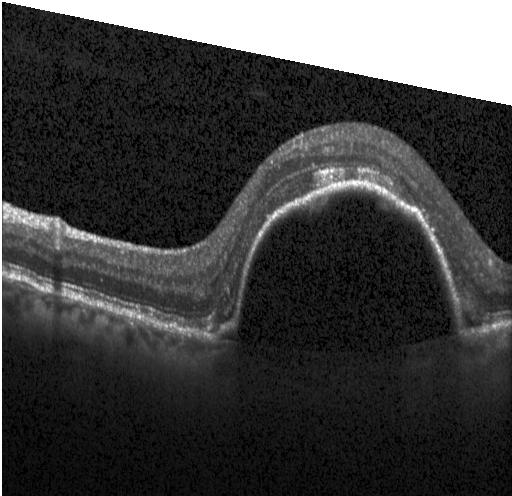 Macular OCT demonstrating a choroidal neovascular membrane.